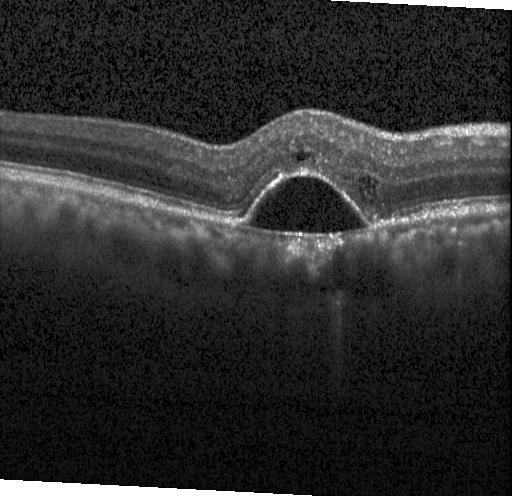

A choroidal neovascular membrane.